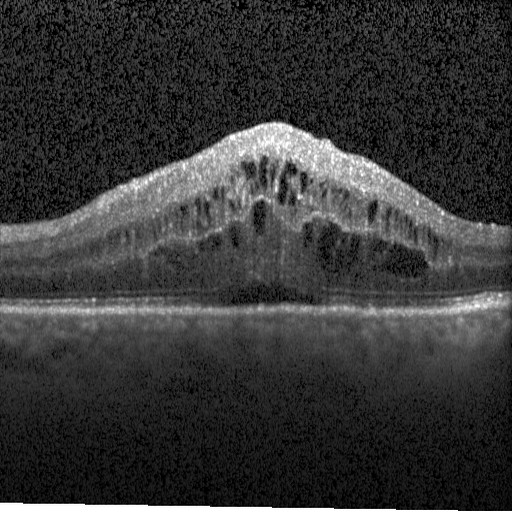

Instrument: Heidelberg Spectralis · retinal OCT cross-section · SD-OCT · centered on the fovea. Finding: diabetic macular edema (DME).